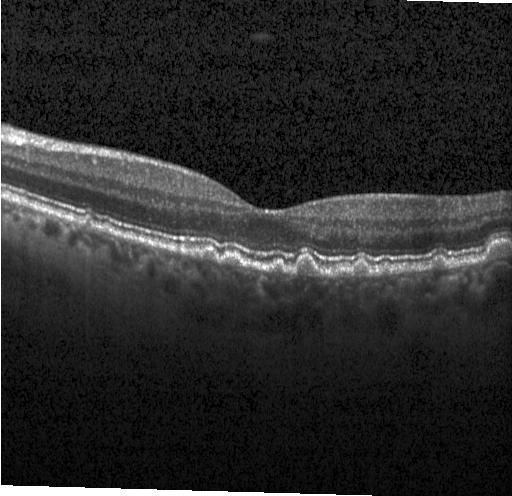

OCT B-scan
Diagnosis: multiple drusen.